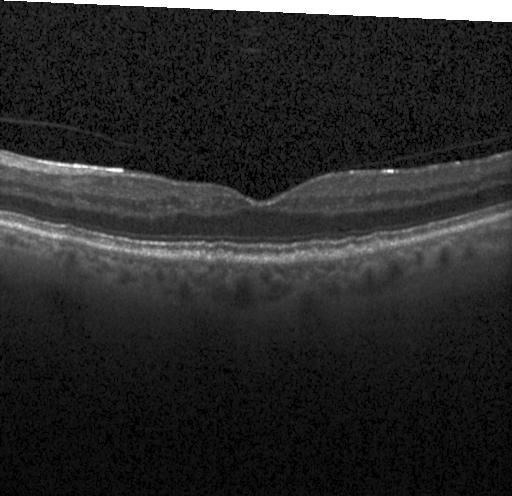
Multiple drusen.